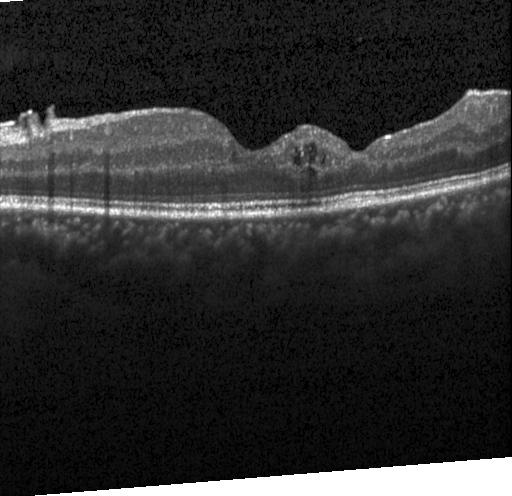
Acquired on a Heidelberg Spectralis; OCT B-scan
Impression: diabetic macular edema.